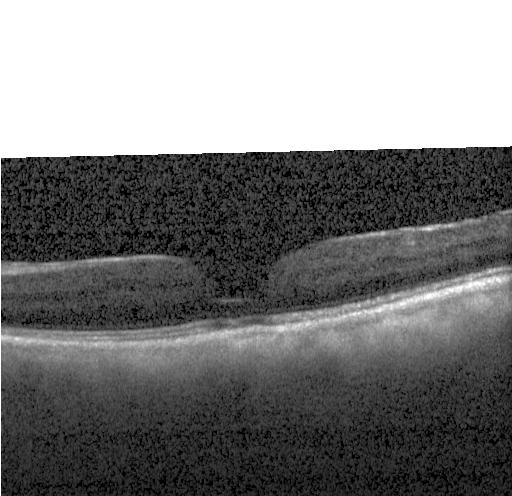 Retinal OCT cross-section showing no choroidal neovascularization, diabetic macular edema, or drusen.